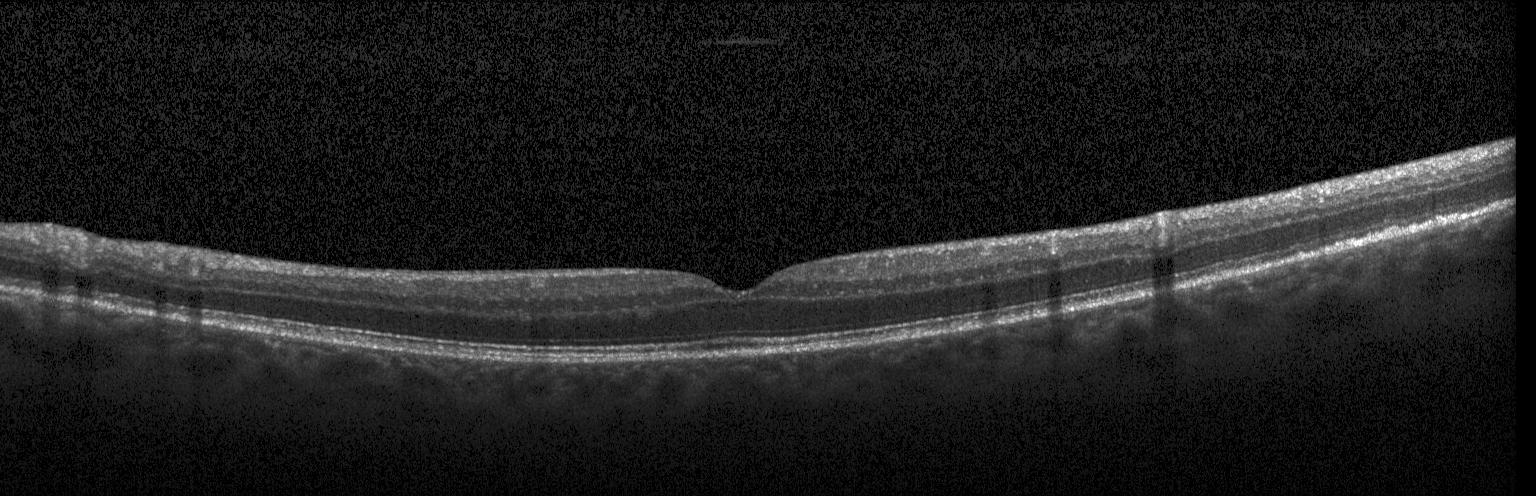 Dx: neither CNV, DME, nor drusen.